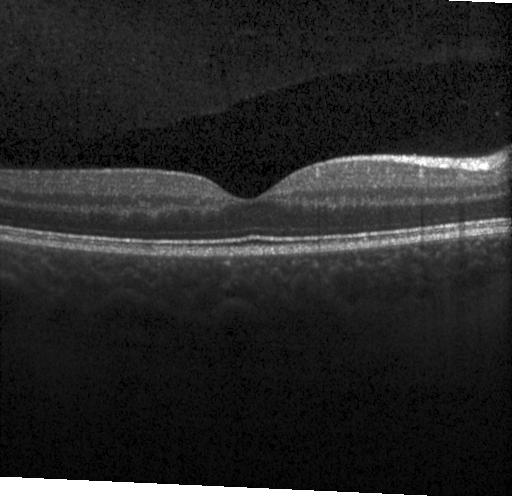 OCT B-scan — Diagnosis: no choroidal neovascularization, no diabetic macular edema, and no drusen.